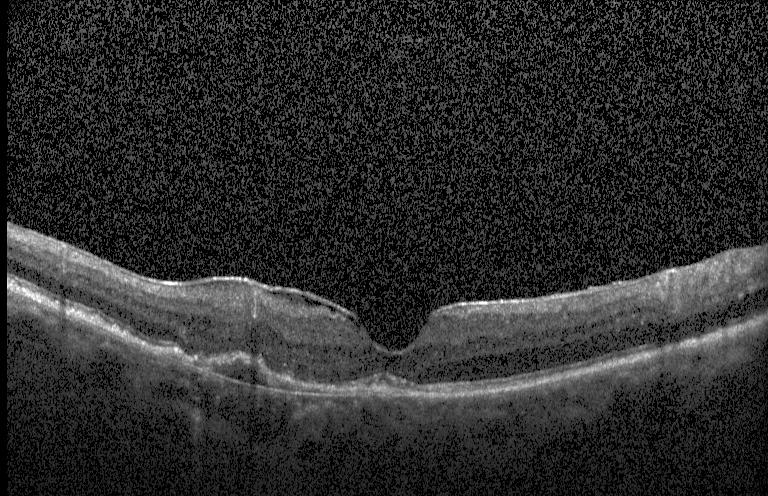 OCT line scan. Horizontal scan through the fovea. Heidelberg Spectralis OCT system. Spectral-domain optical coherence tomography
Diagnosis: choroidal neovascularization (CNV).